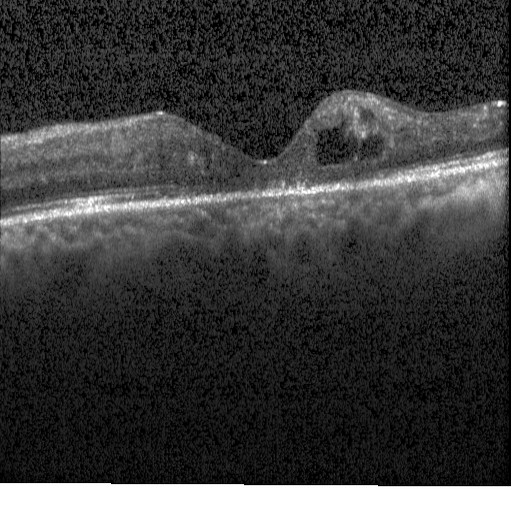

OCT scan showing diabetic macular edema (DME).